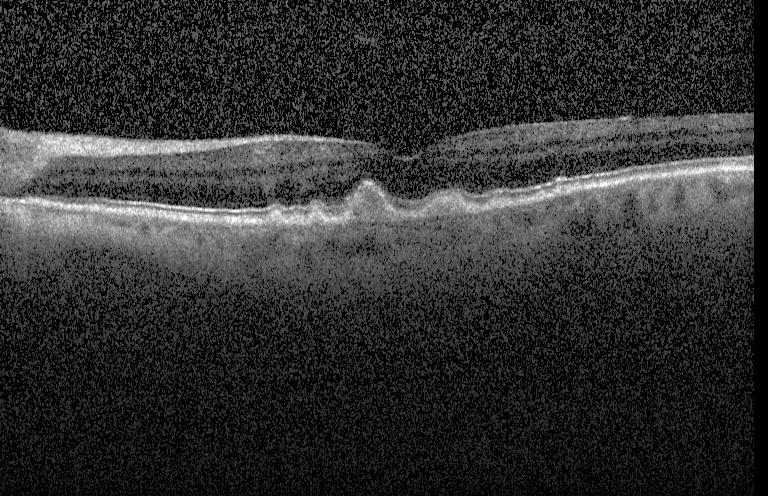
OCT line scan. Instrument: Heidelberg Spectralis
This B-scan demonstrates multiple drusen.